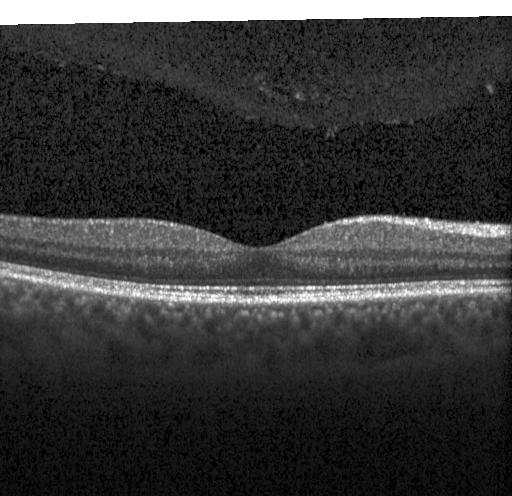

Dx: neither choroidal neovascularization, diabetic macular edema, nor drusen.